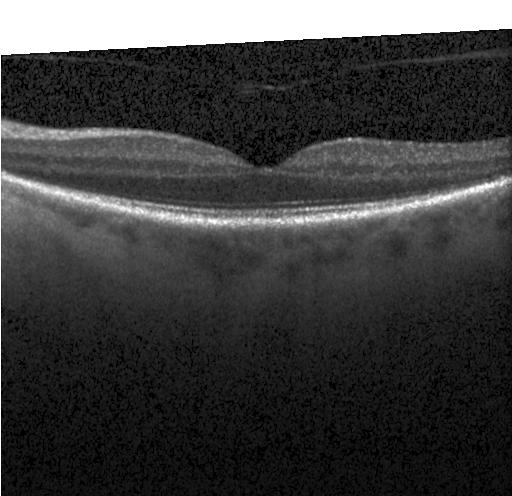 Optical coherence tomography scan · SD-OCT. Finding: neither choroidal neovascularization, diabetic macular edema, nor drusen.